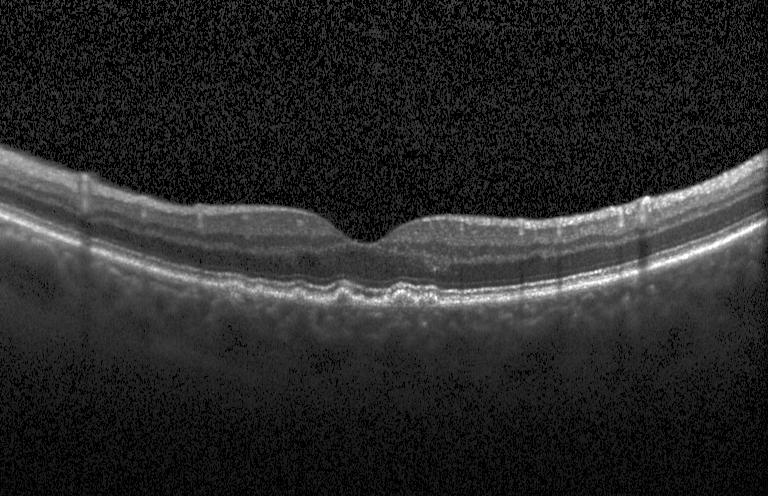
Optical coherence tomography B-scan; through the macula; acquired on a Heidelberg Spectralis.
This B-scan demonstrates sub-RPE drusenoid deposits.